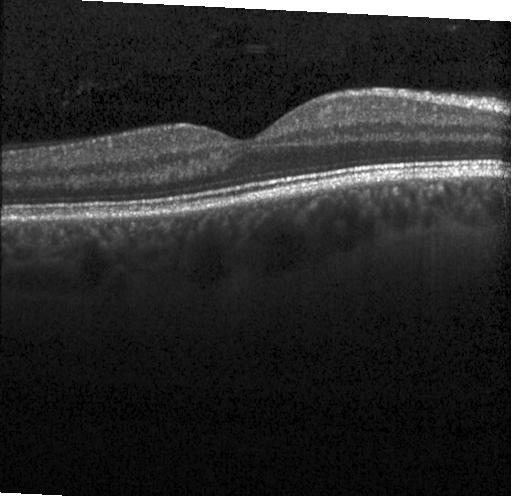
OCT scan showing no choroidal neovascularization, diabetic macular edema, or drusen.